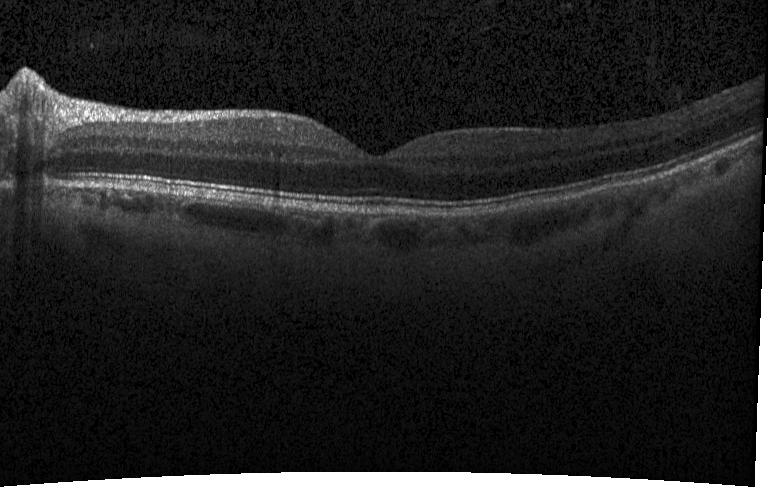
Retinal OCT cross-section showing no choroidal neovascularization, no diabetic macular edema, and no drusen.